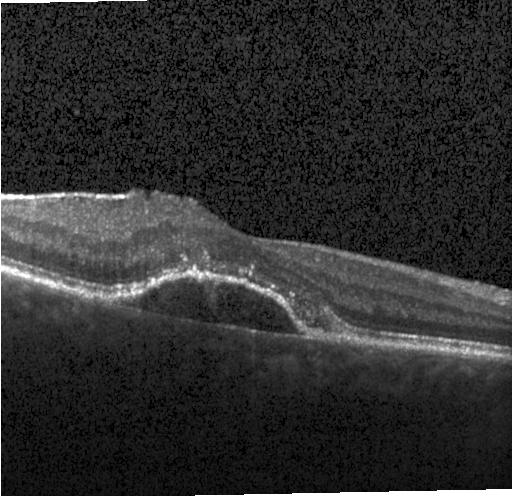 OCT line scan. Macular OCT: CNV.